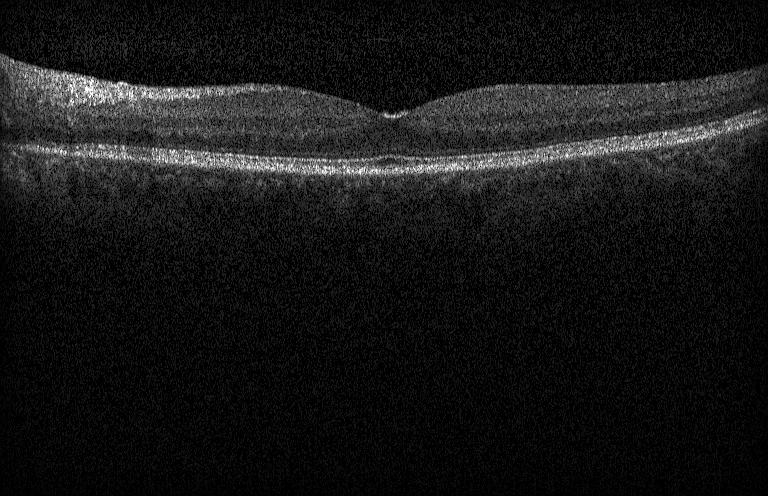

OCT finding: no evidence of CNV, DME, or drusen.